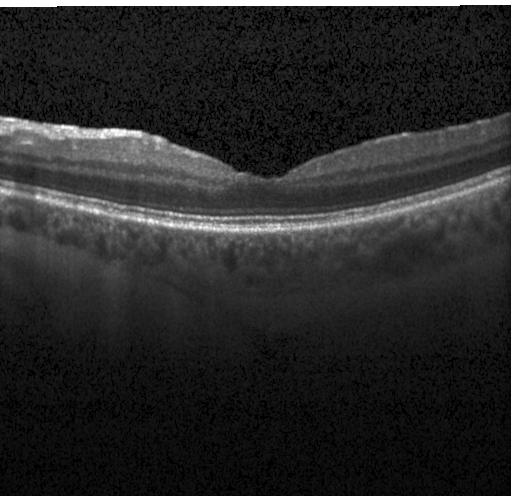
Optical coherence tomography B-scan. Heidelberg Spectralis. SD-OCT
No evidence of choroidal neovascularization, diabetic macular edema, or drusen.